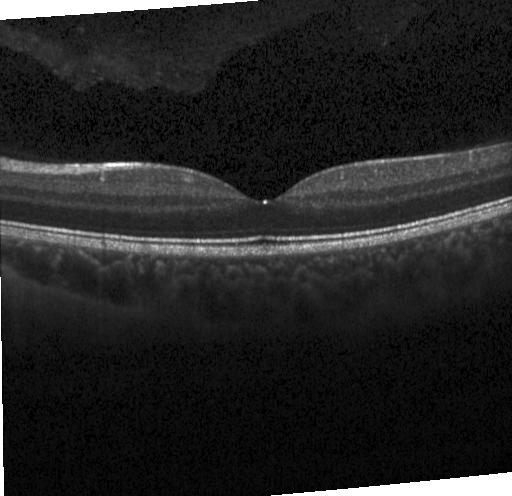

Diagnosis: no evidence of choroidal neovascularization, diabetic macular edema, or drusen.